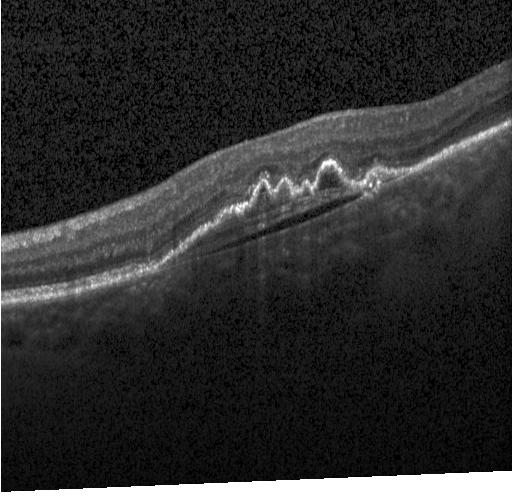
SD-OCT · Heidelberg Spectralis OCT system · centered on the fovea · OCT B-scan — Diagnosis: choroidal neovascularization (CNV).